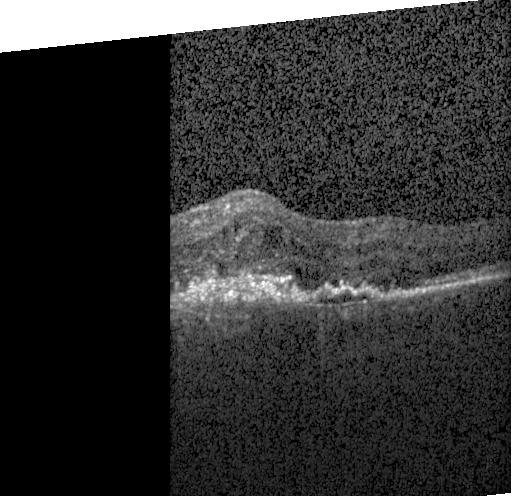

Heidelberg Spectralis · horizontal scan through the fovea · optical coherence tomography B-scan · SD-OCT.
Choroidal neovascularization (CNV).